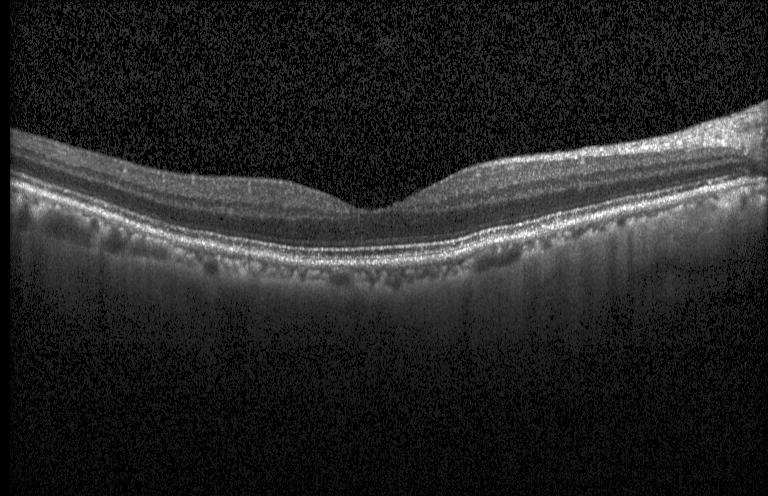 Optical coherence tomography scan; SD-OCT. Finding: no evidence of choroidal neovascularization, diabetic macular edema, or drusen.